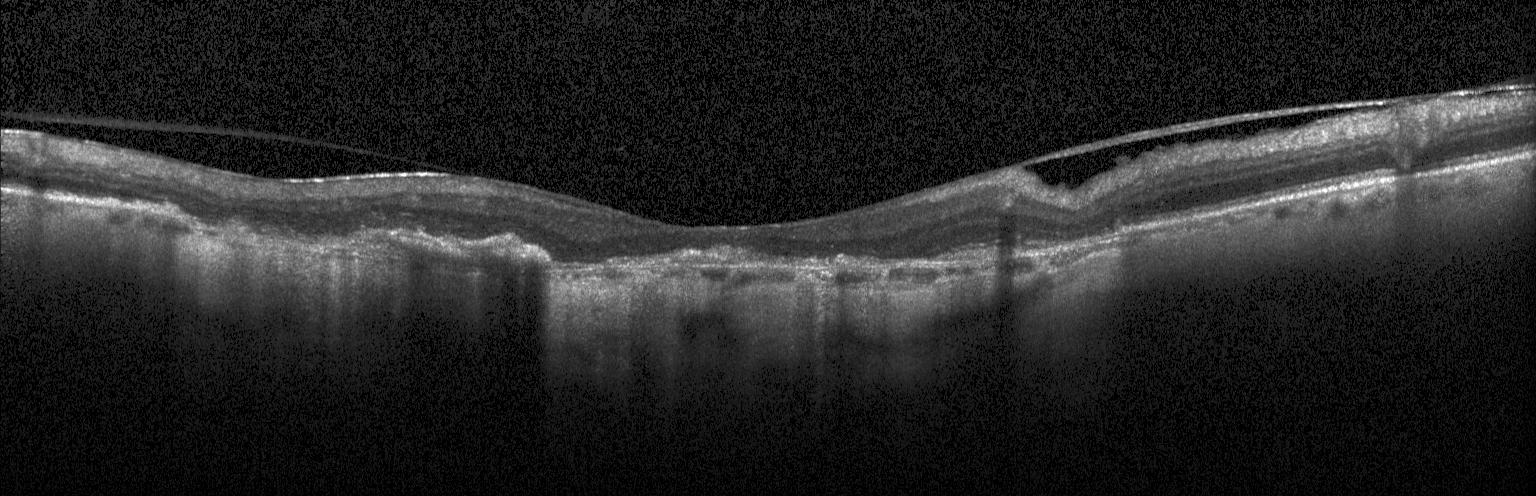
Spectral-domain OCT B-scan: a choroidal neovascular membrane.